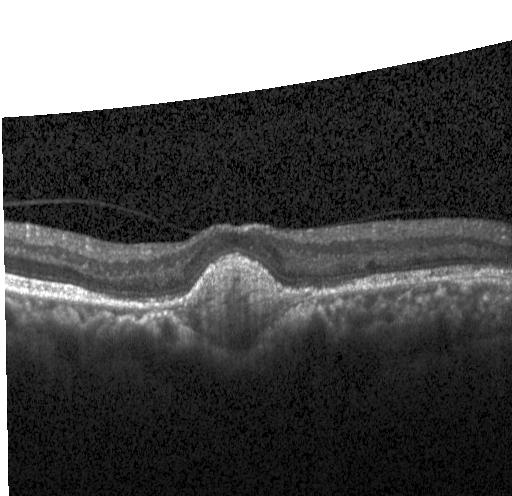 This B-scan demonstrates choroidal neovascularization (CNV).